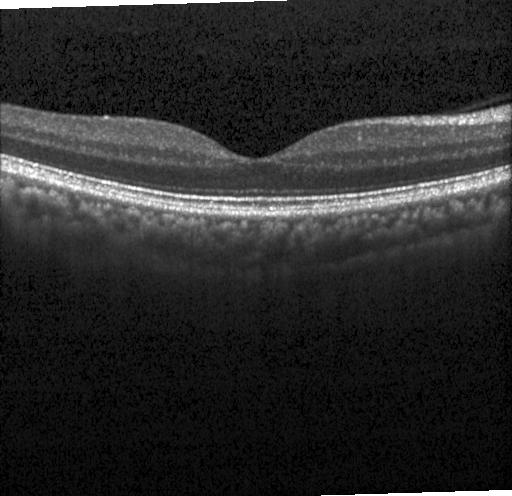

Heidelberg Spectralis · spectral-domain optical coherence tomography · retinal OCT B-scan · through the macula.
Impression: neither CNV, DME, nor drusen.